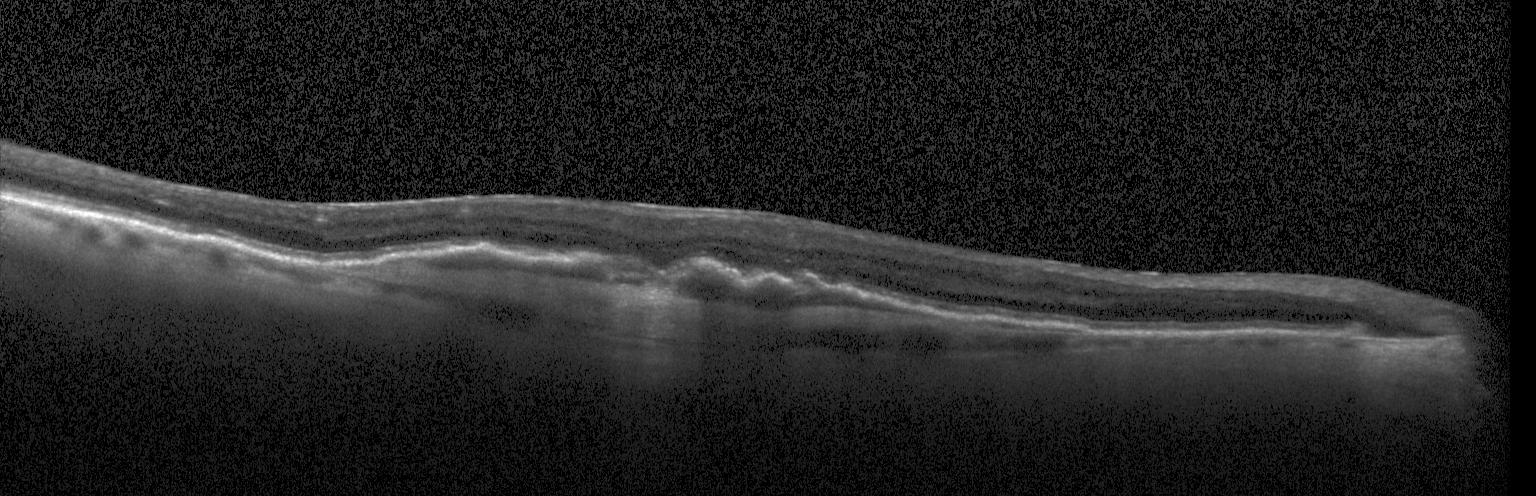

OCT scan showing a choroidal neovascular membrane.